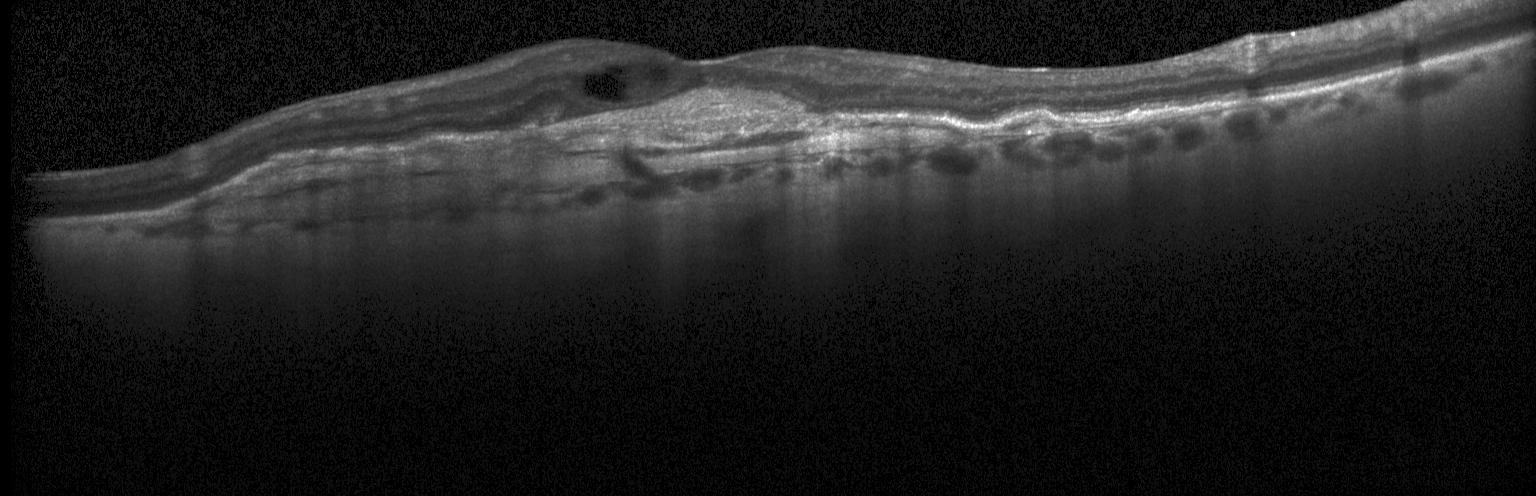
Centered on the fovea, spectral-domain OCT, optical coherence tomography B-scan, acquired on a Heidelberg Spectralis
Assessment: CNV.